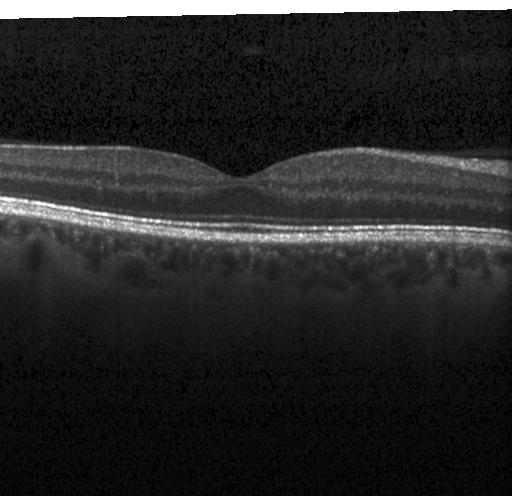
OCT B-scan
Impression: no evidence of choroidal neovascularization, diabetic macular edema, or drusen.